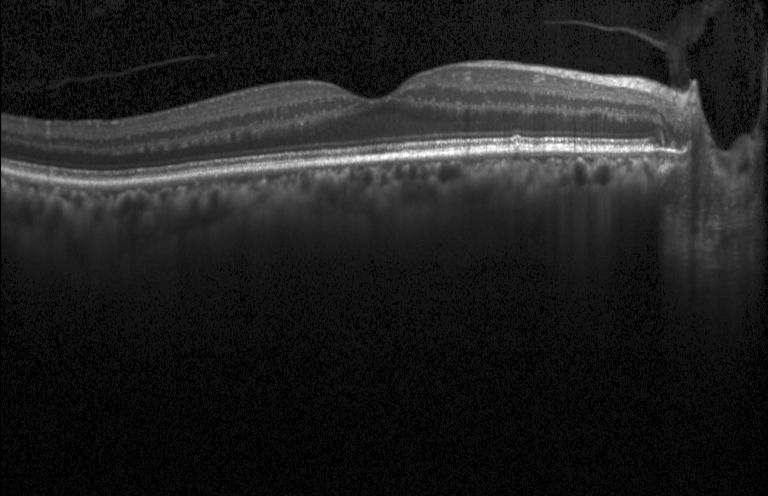
This B-scan demonstrates no choroidal neovascularization, diabetic macular edema, or drusen.